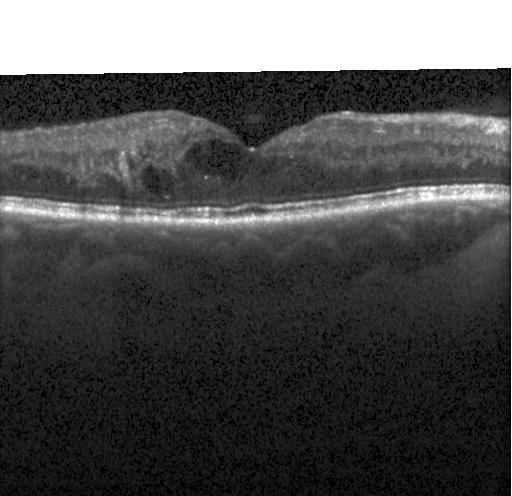

The scan shows diabetic macular edema.